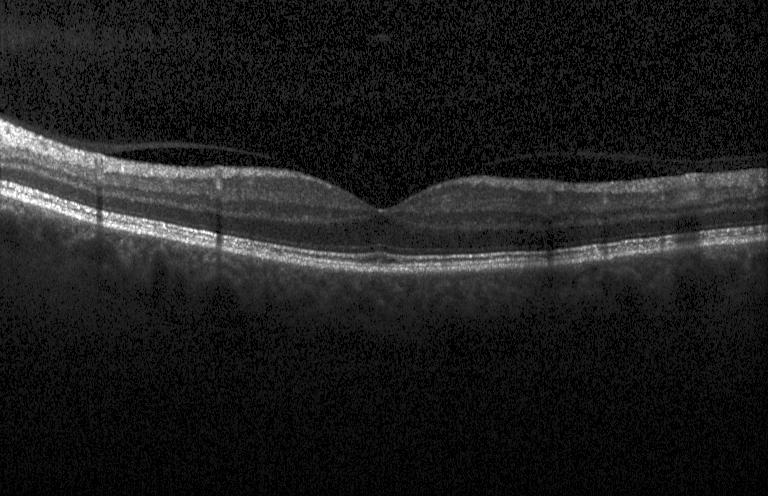 Heidelberg Spectralis OCT system. Horizontal scan through the fovea. Optical coherence tomography scan. SD-OCT. The scan shows no choroidal neovascularization, diabetic macular edema, or drusen.